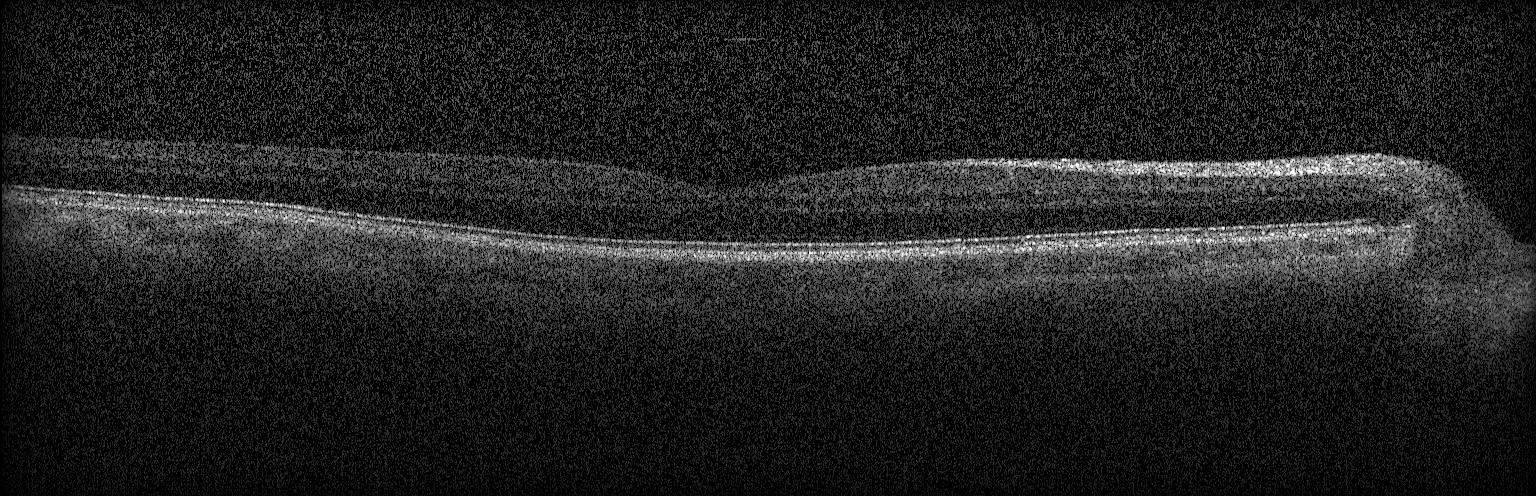
Dx: no choroidal neovascularization, no diabetic macular edema, and no drusen.